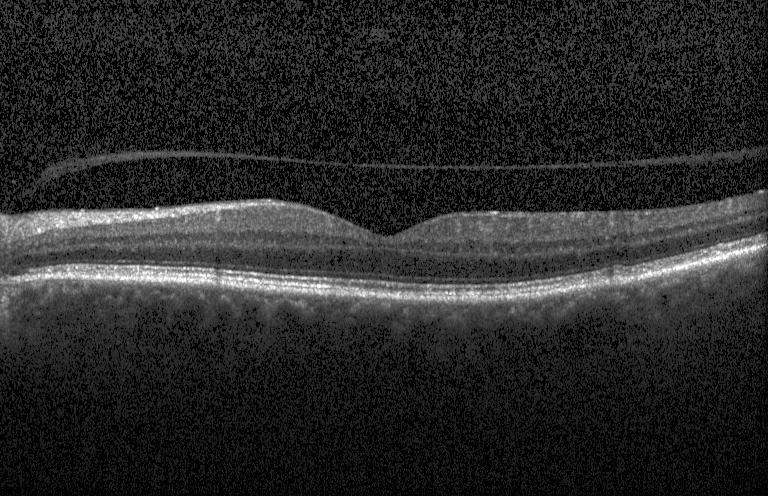

OCT line scan. No evidence of CNV, DME, or drusen.